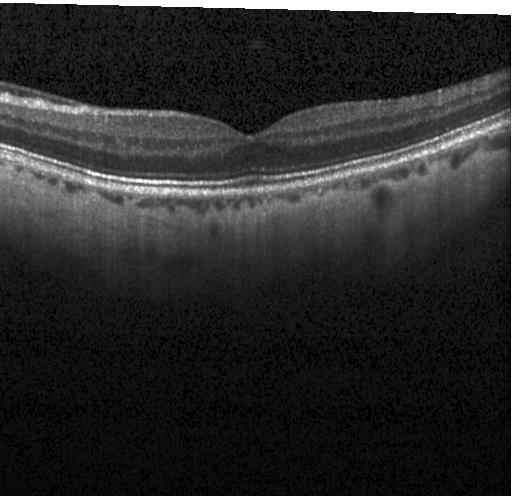
Through the macula, OCT B-scan — Macular OCT: no choroidal neovascularization, diabetic macular edema, or drusen.